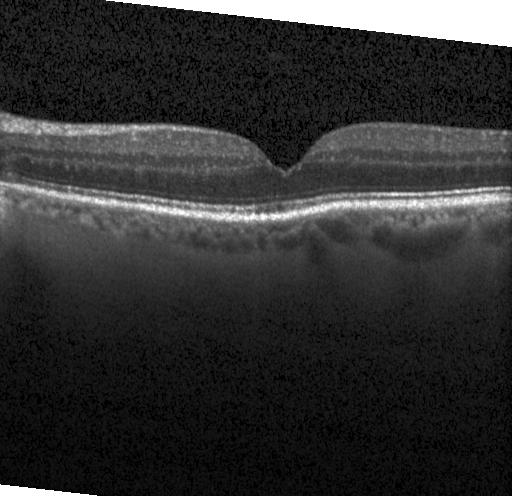 Spectral-domain OCT, retinal OCT cross-section
The scan shows no choroidal neovascularization, diabetic macular edema, or drusen.